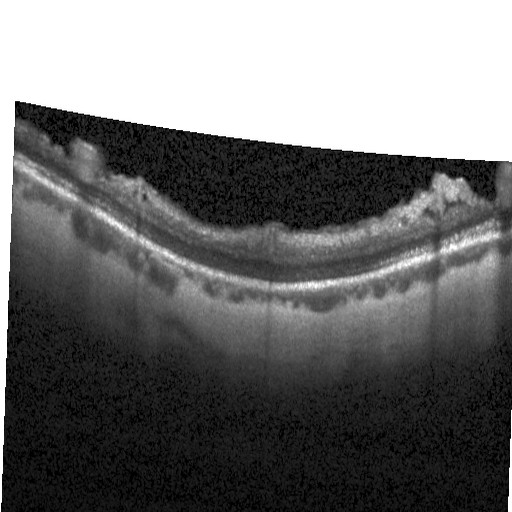 Macular OCT demonstrating diabetic macular edema.